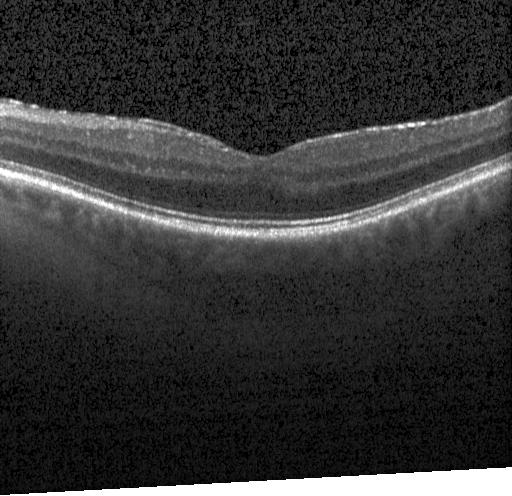 Instrument: Heidelberg Spectralis, OCT line scan, spectral-domain OCT
Impression: no choroidal neovascularization, diabetic macular edema, or drusen.